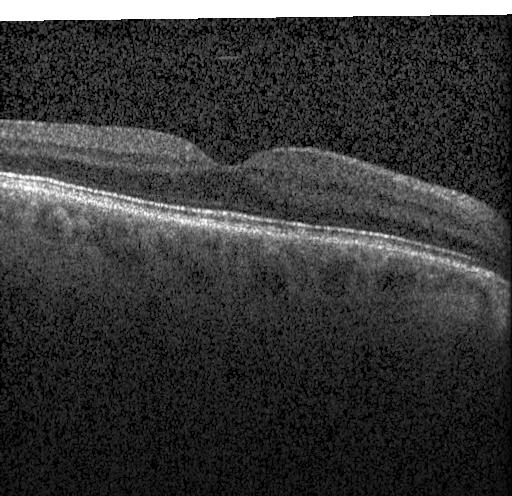
Finding: no evidence of choroidal neovascularization, diabetic macular edema, or drusen.